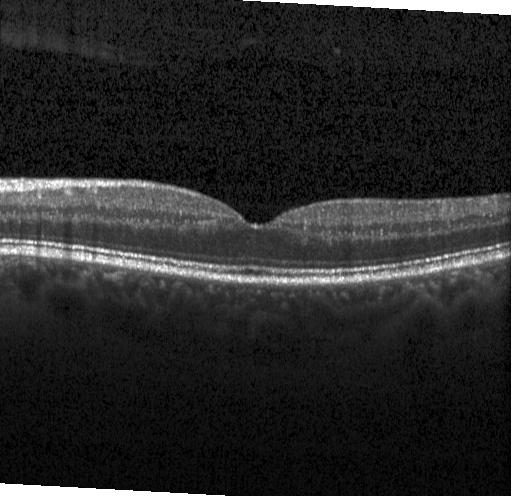

Macular scan · SD-OCT · retinal OCT B-scan · acquired on a Heidelberg Spectralis — Impression: no CNV, no DME, and no drusen.